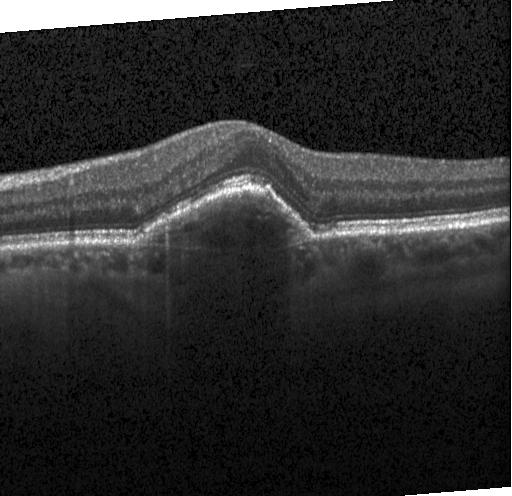
Spectral-domain optical coherence tomography. Retinal OCT cross-section. Centered on the fovea. OCT finding: choroidal neovascularization.